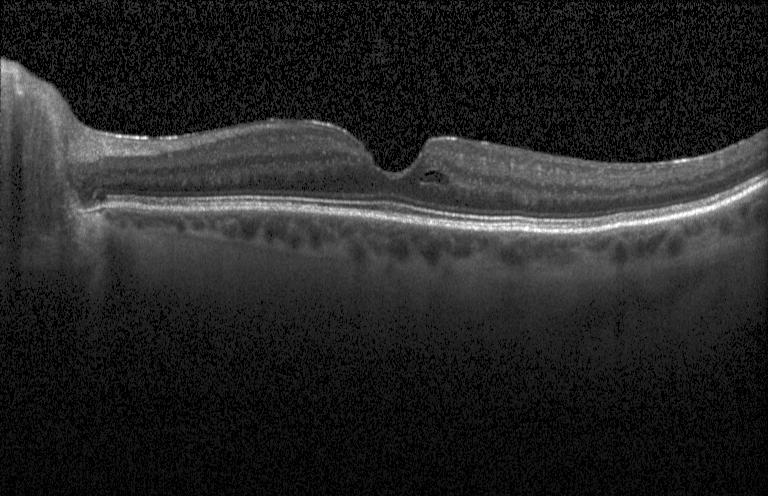

Spectral-domain OCT. Fovea-centered. Acquired on a Heidelberg Spectralis. OCT B-scan — Finding: diabetic macular edema.